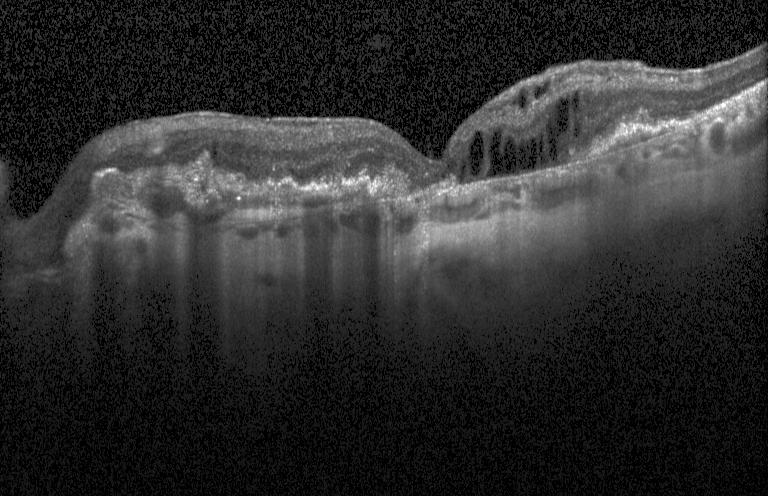
Fovea-centered; OCT B-scan; SD-OCT
Assessment: choroidal neovascularization (CNV).